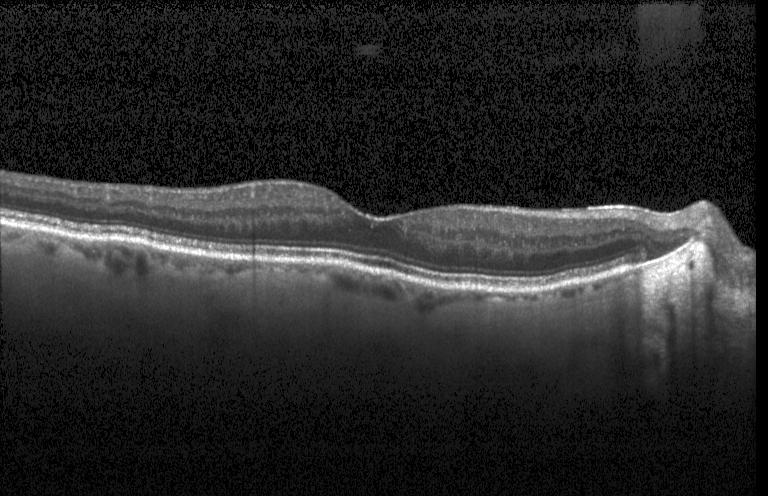
OCT line scan — This B-scan demonstrates no evidence of choroidal neovascularization, diabetic macular edema, or drusen.